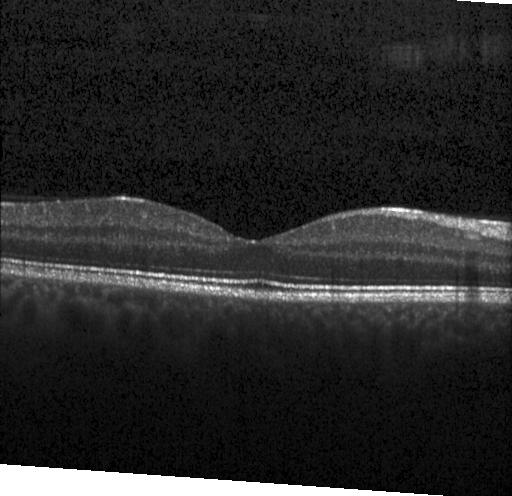
OCT line scan · horizontal scan through the fovea.
No choroidal neovascularization, diabetic macular edema, or drusen.